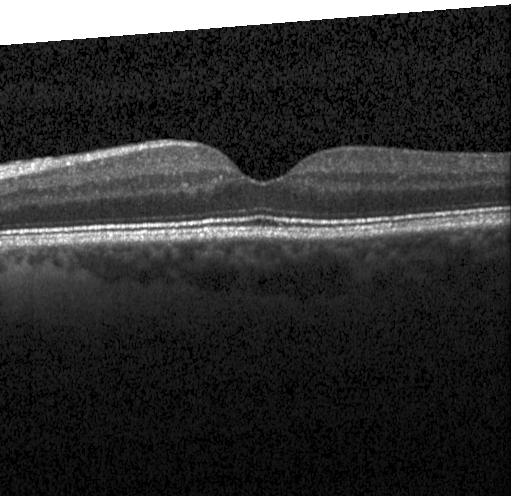 OCT line scan
OCT finding: no choroidal neovascularization, diabetic macular edema, or drusen.